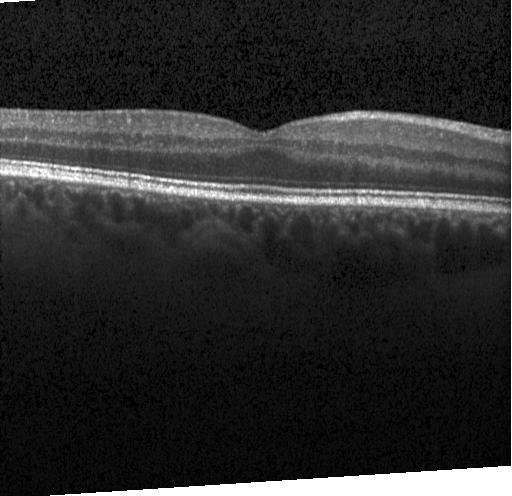 OCT finding: no evidence of choroidal neovascularization, diabetic macular edema, or drusen.